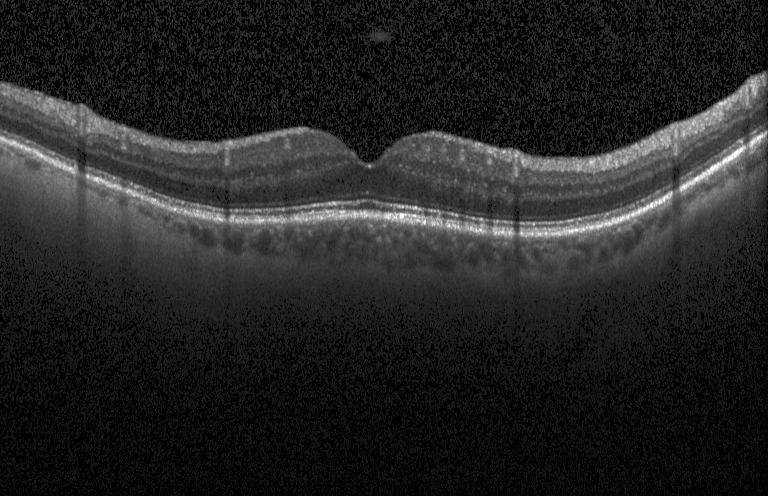
Macular OCT demonstrating no evidence of CNV, DME, or drusen.